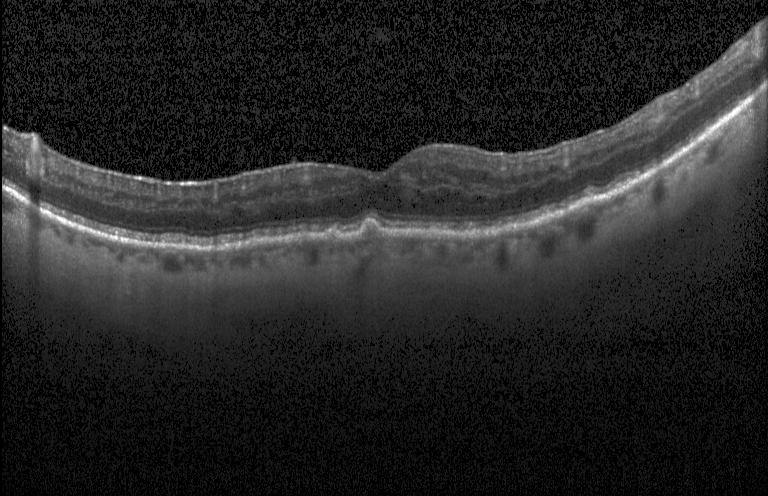 Spectral-domain optical coherence tomography. Macular scan. Instrument: Heidelberg Spectralis. Optical coherence tomography scan — This B-scan demonstrates sub-RPE drusenoid deposits.